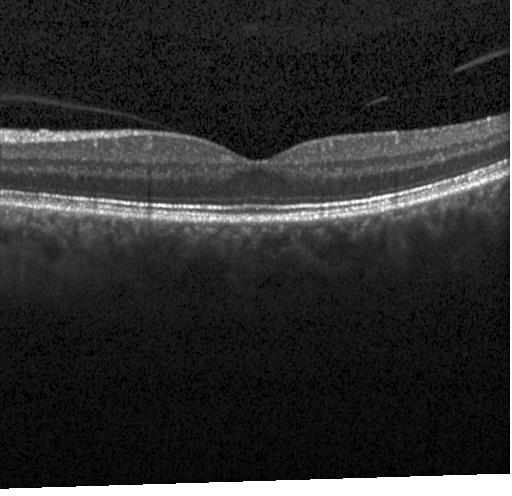 Retinal OCT B-scan; fovea-centered; spectral-domain OCT; instrument: Heidelberg Spectralis — Impression: no CNV, DME, or drusen.